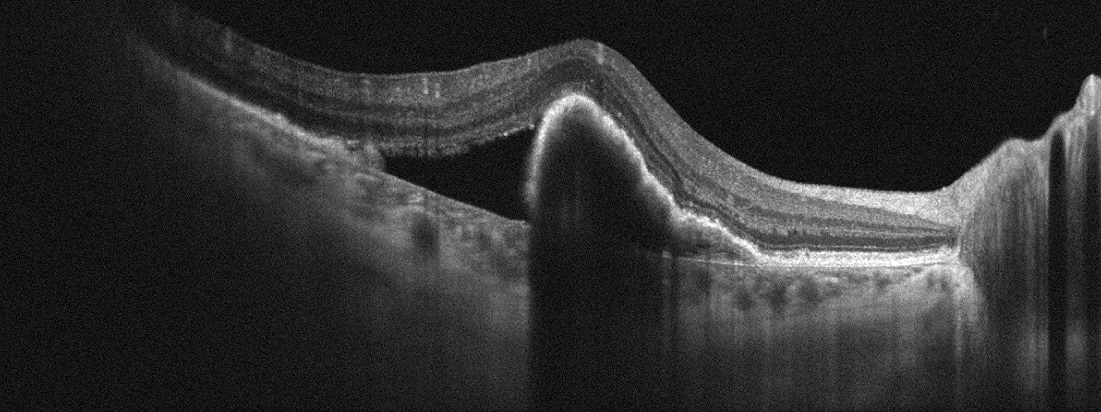 Macular OCT: age-related macular degeneration.